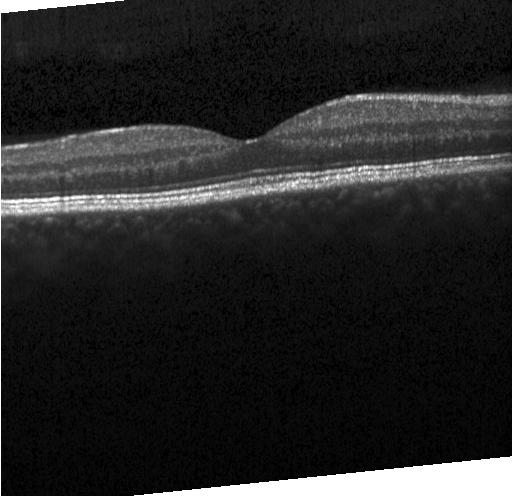 OCT scan showing no choroidal neovascularization, diabetic macular edema, or drusen.